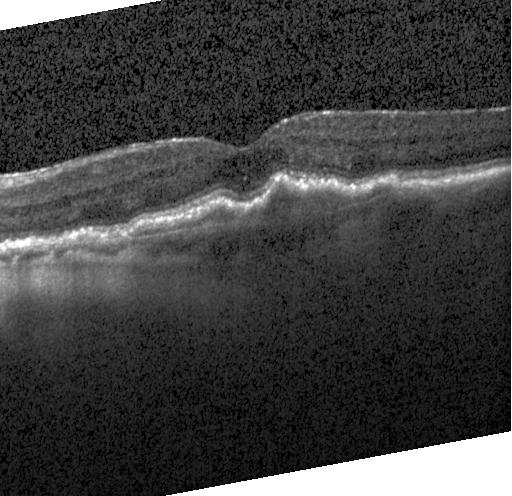
This B-scan demonstrates a choroidal neovascular membrane.